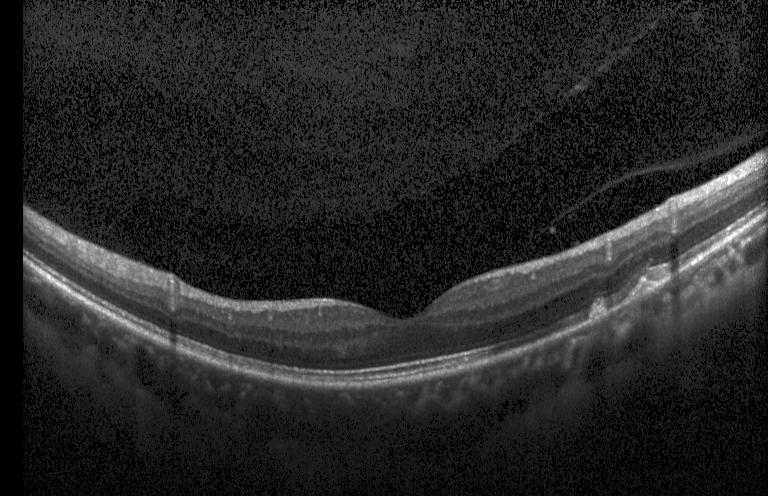

OCT scan showing multiple drusen.